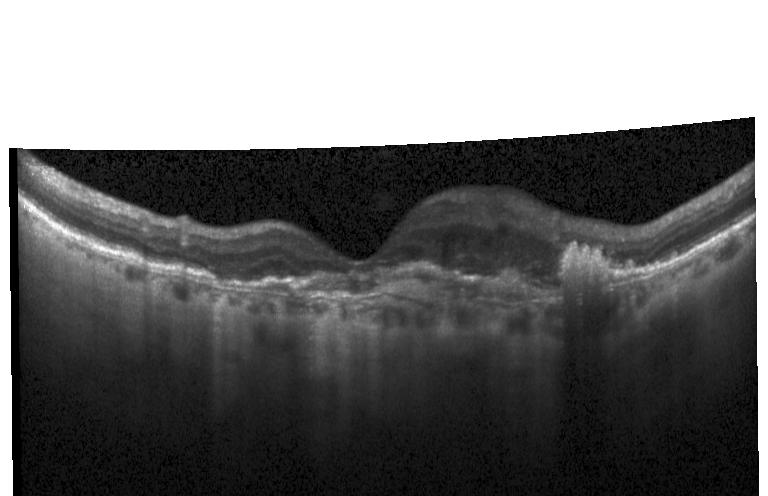 Instrument: Heidelberg Spectralis. SD-OCT. Retinal OCT B-scan. Fovea-centered.
OCT finding: choroidal neovascularization (CNV).